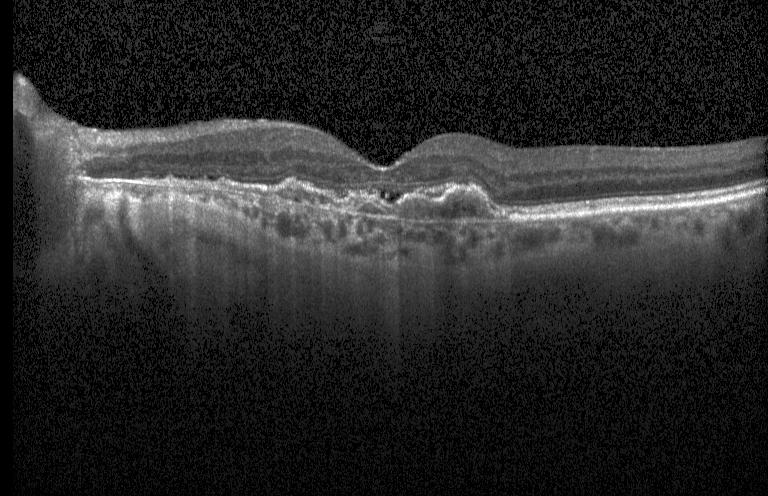

Macular OCT: CNV.